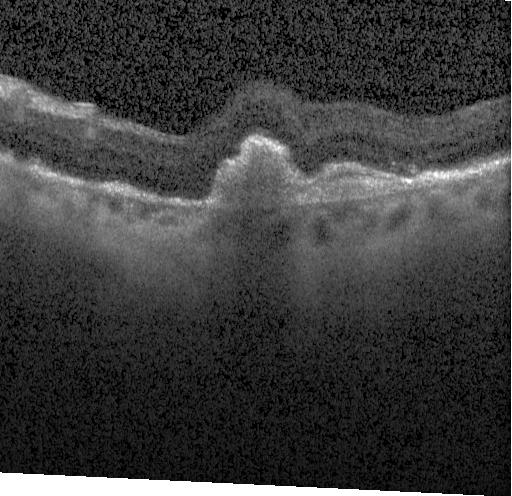 Optical coherence tomography scan.
Impression: a choroidal neovascular membrane.